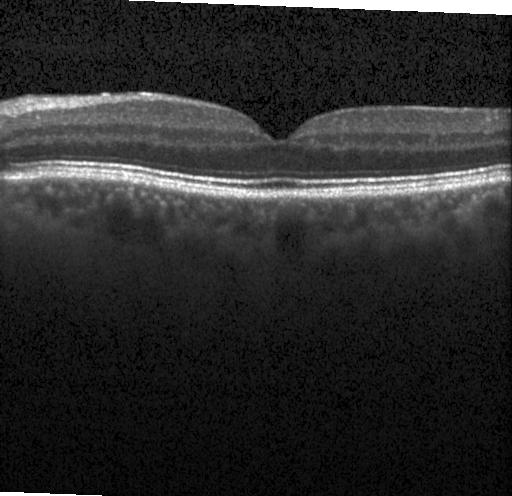 Spectral-domain OCT B-scan: neither CNV, DME, nor drusen.